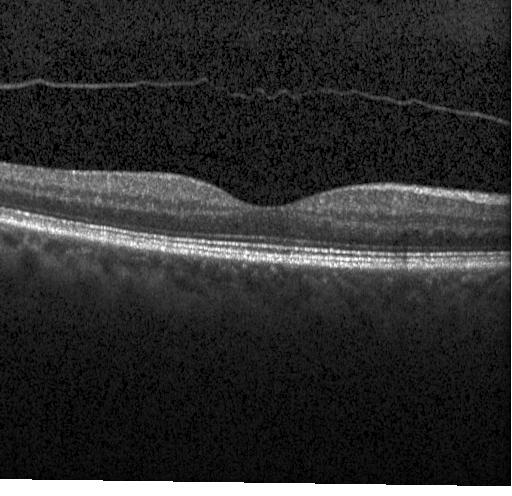

Heidelberg Spectralis; retinal OCT cross-section; fovea-centered.
Impression: no CNV, no DME, and no drusen.